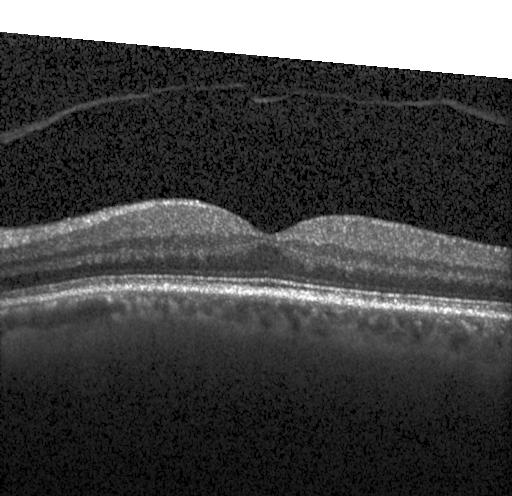
Retinal OCT B-scan. Diagnosis: no choroidal neovascularization, diabetic macular edema, or drusen.